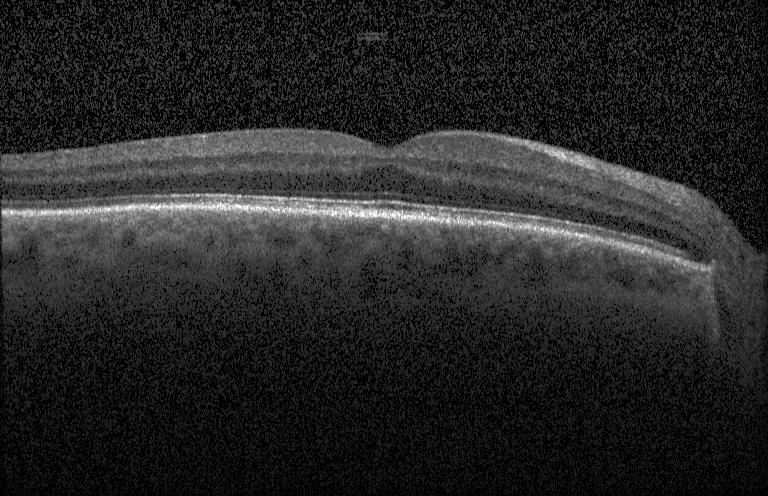 Spectral-domain optical coherence tomography; retinal OCT B-scan. Macular OCT: no evidence of choroidal neovascularization, diabetic macular edema, or drusen.